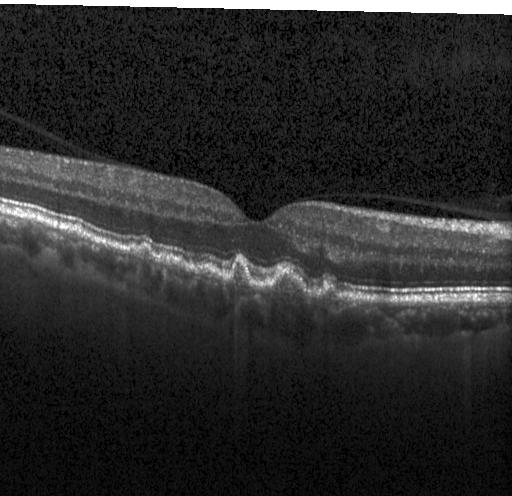 Fovea-centered, OCT line scan, instrument: Heidelberg Spectralis, spectral-domain optical coherence tomography — Impression: sub-RPE drusenoid deposits.